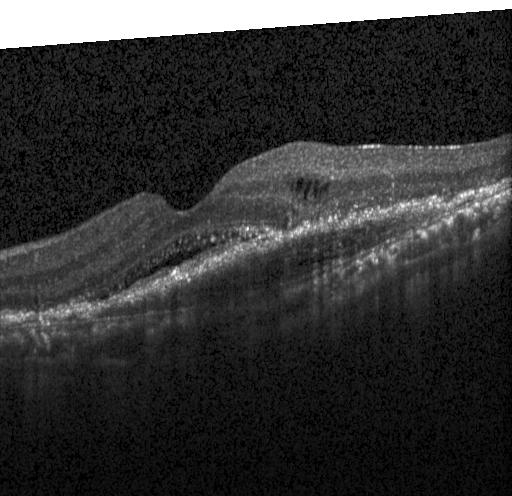 OCT line scan · SD-OCT
Macular OCT: a choroidal neovascular membrane.